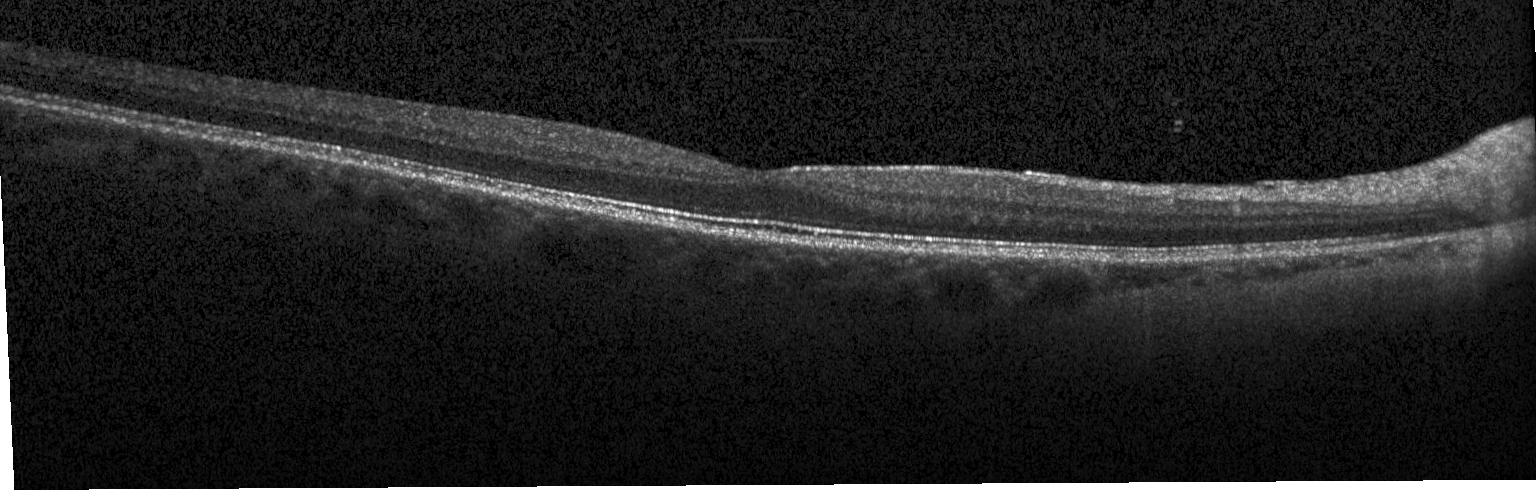
OCT B-scan showing no evidence of choroidal neovascularization, diabetic macular edema, or drusen.